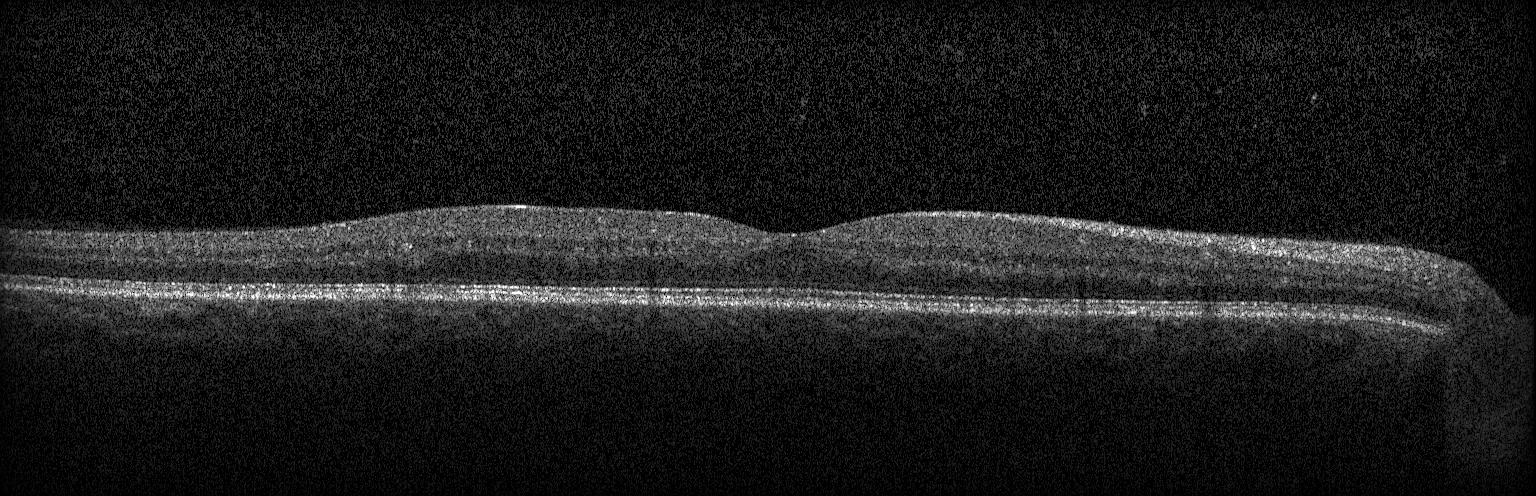 Fovea-centered, retinal OCT cross-section.
Finding: no evidence of CNV, DME, or drusen.